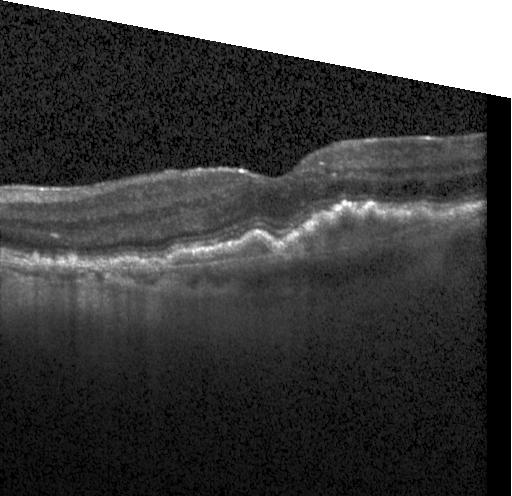 OCT B-scan showing CNV.